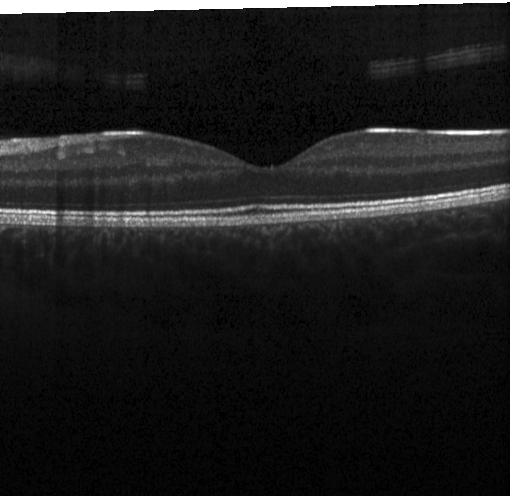

Finding: no CNV, no DME, and no drusen.